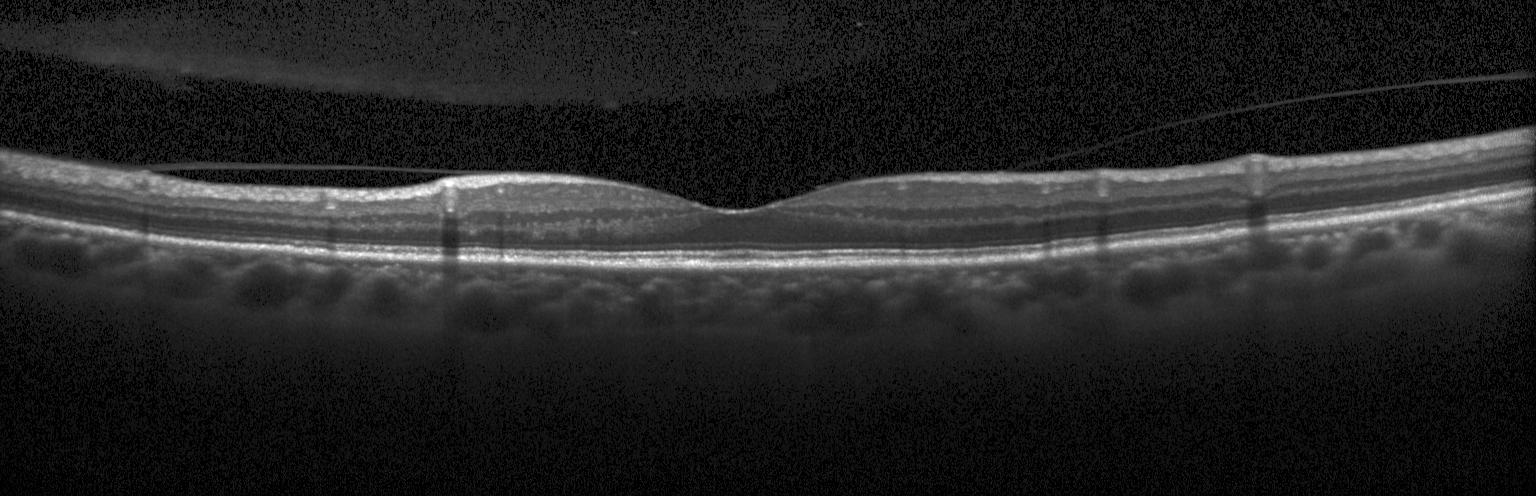 OCT scan showing no choroidal neovascularization, diabetic macular edema, or drusen.